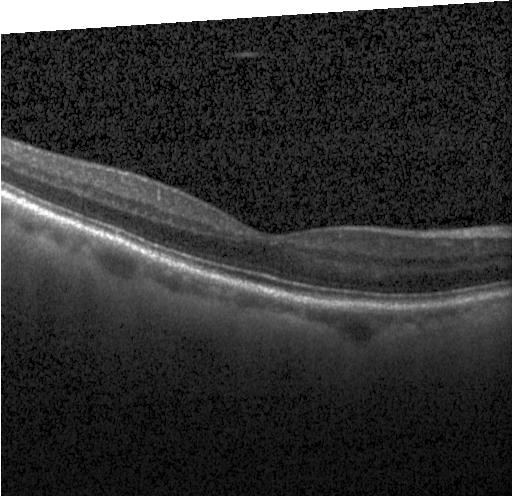

Retinal OCT B-scan. Assessment: no evidence of CNV, DME, or drusen.